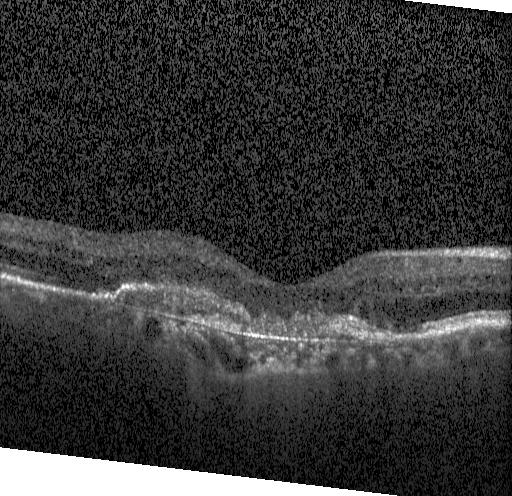

Through the macula · acquired on a Heidelberg Spectralis · retinal OCT cross-section.
This B-scan demonstrates CNV.